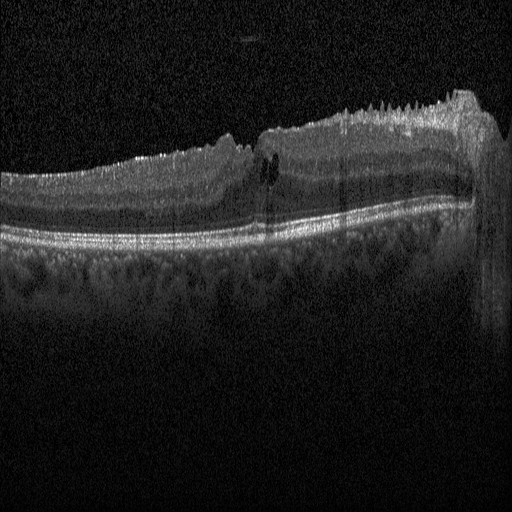 Assessment: diabetic macular edema.